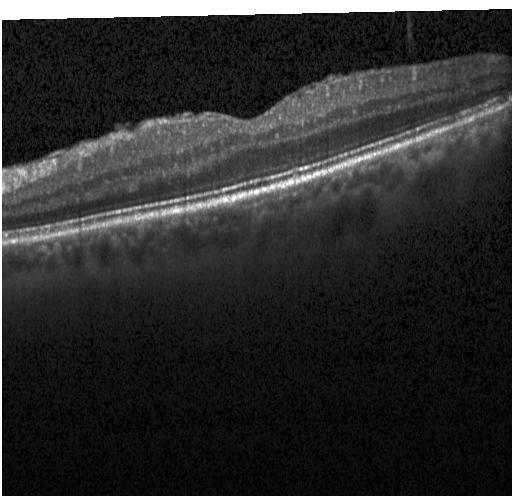

Dx: no choroidal neovascularization, diabetic macular edema, or drusen.